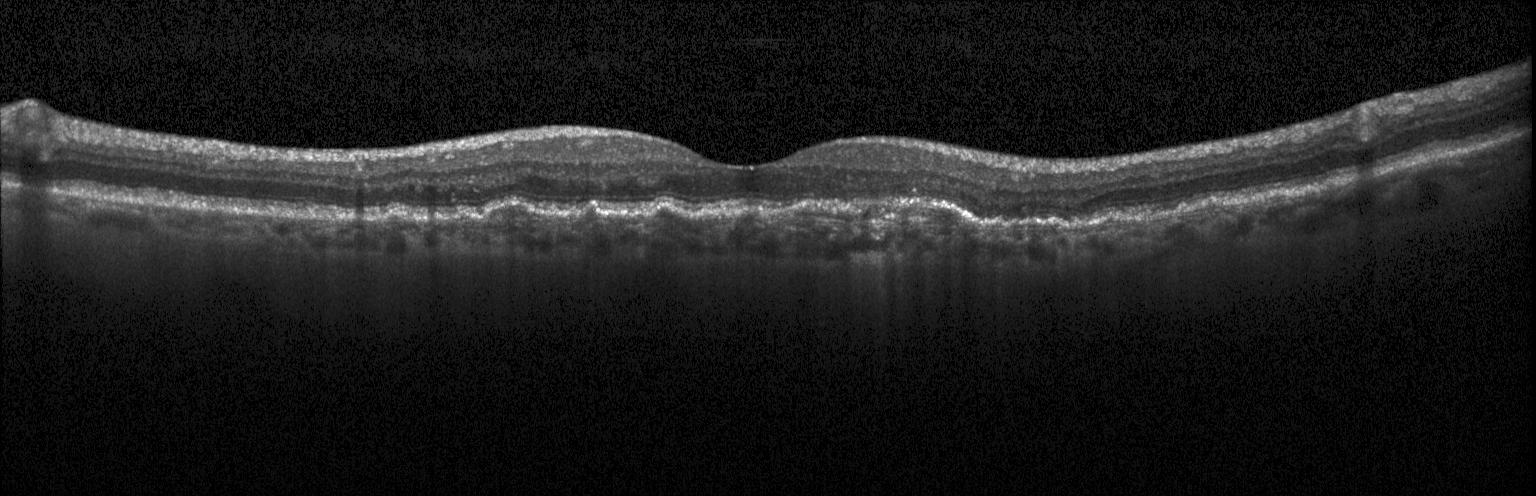
Instrument: Heidelberg Spectralis, centered on the fovea, SD-OCT, optical coherence tomography B-scan.
Diagnosis: choroidal neovascularization.